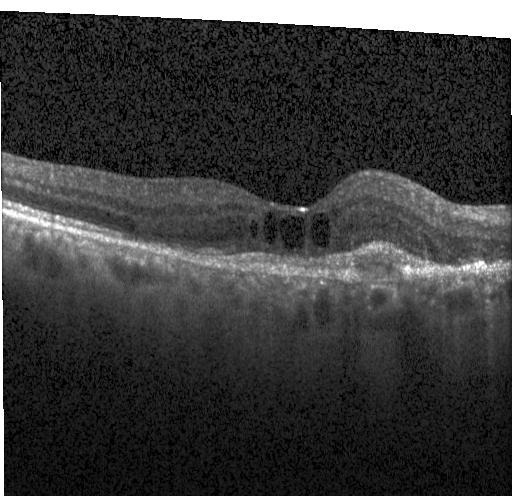 Spectral-domain optical coherence tomography · acquired on a Heidelberg Spectralis · retinal OCT B-scan
OCT finding: CNV.